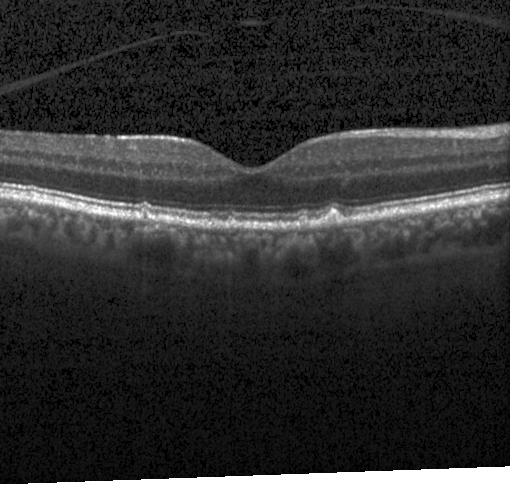
OCT B-scan; acquired on a Heidelberg Spectralis; spectral-domain optical coherence tomography — Finding: drusen.